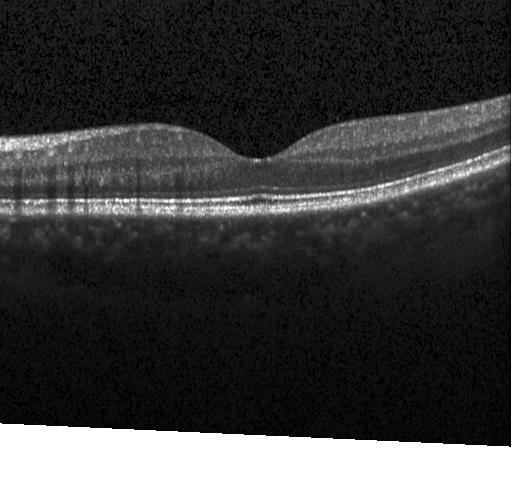
Optical coherence tomography B-scan.
Diagnosis: no choroidal neovascularization, diabetic macular edema, or drusen.